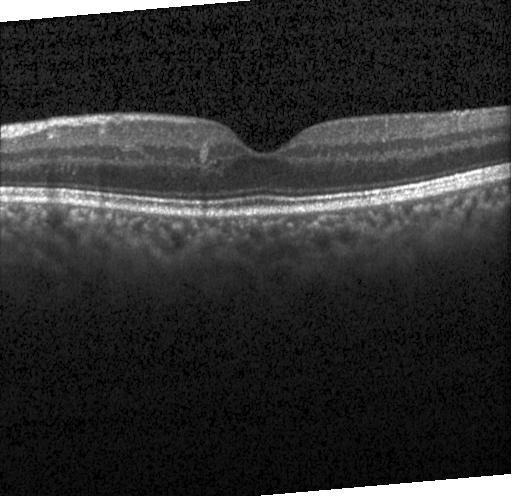 OCT line scan
Impression: neither CNV, DME, nor drusen.